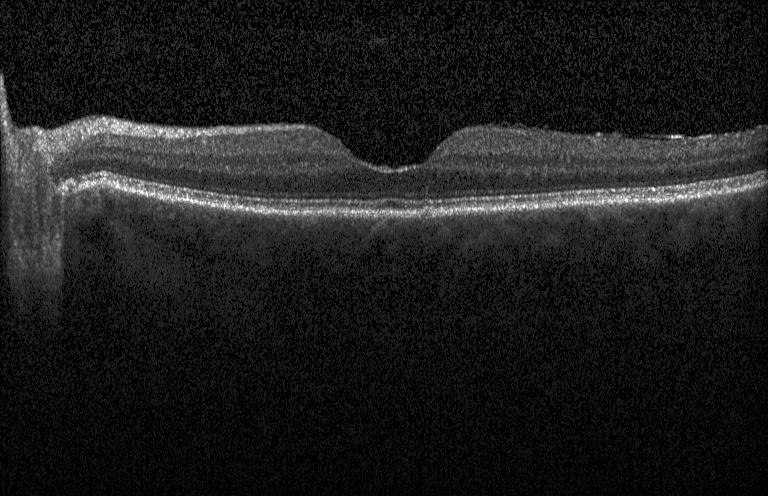
Horizontal scan through the fovea · spectral-domain optical coherence tomography · optical coherence tomography B-scan.
The scan shows no evidence of choroidal neovascularization, diabetic macular edema, or drusen.